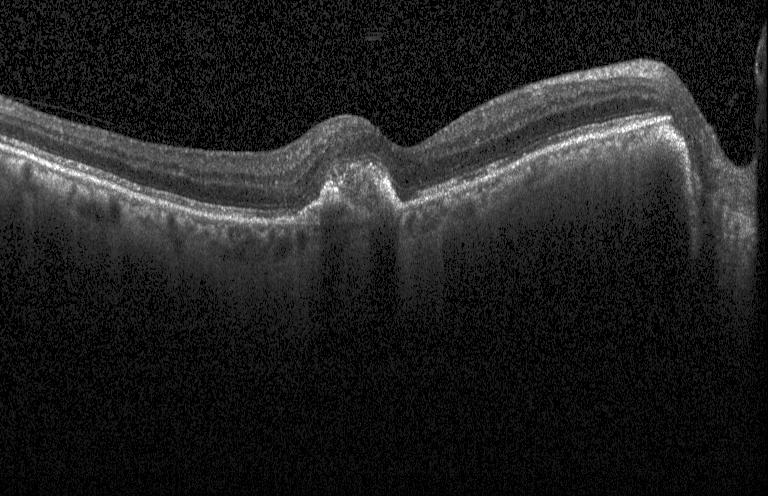 Optical coherence tomography scan — A choroidal neovascular membrane.